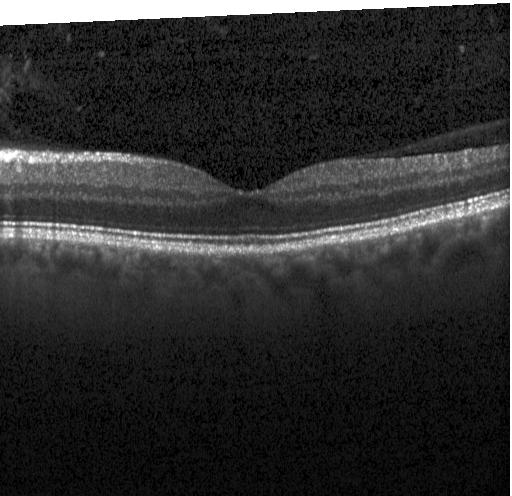
Fovea-centered, Heidelberg Spectralis OCT system, OCT B-scan, spectral-domain optical coherence tomography. This B-scan demonstrates no choroidal neovascularization, diabetic macular edema, or drusen.